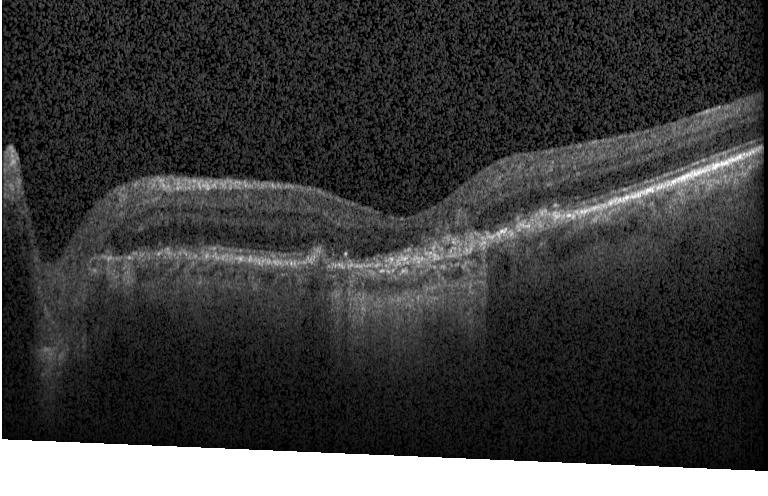

Fovea-centered, optical coherence tomography B-scan — Assessment: a choroidal neovascular membrane.